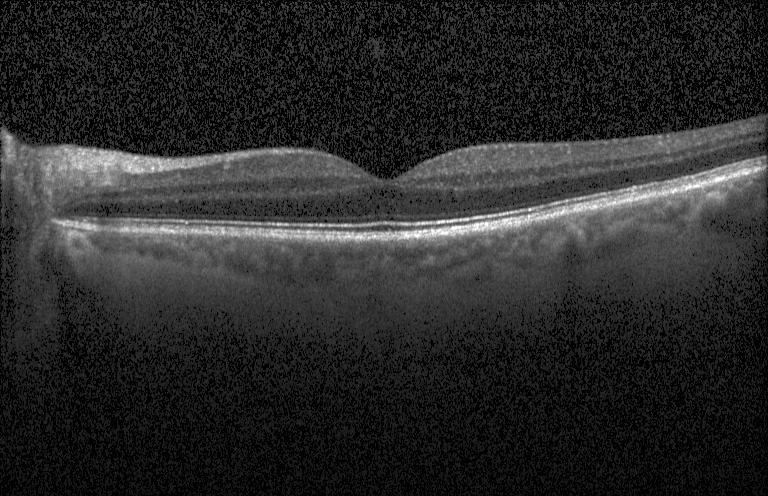

Macular OCT: neither CNV, DME, nor drusen.